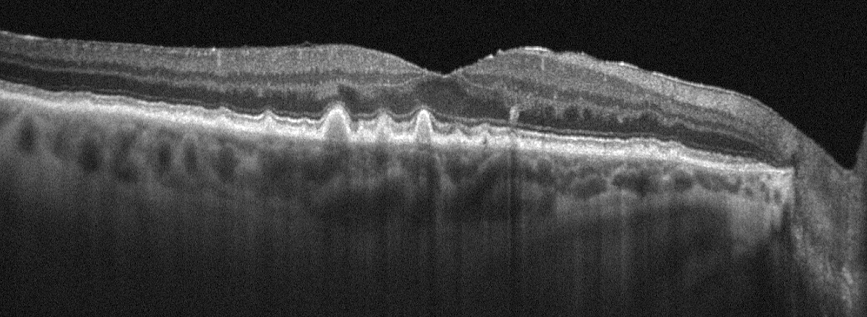 Finding: AMD.